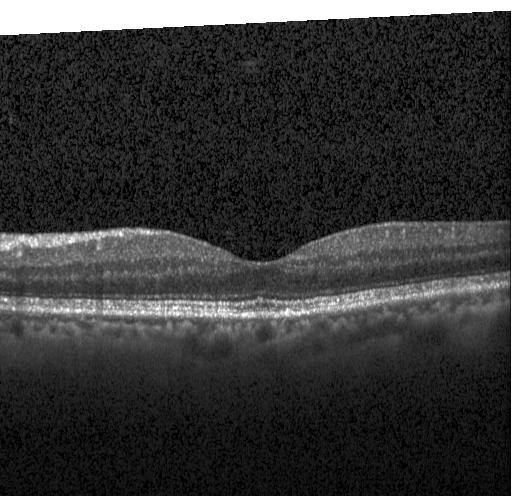
Heidelberg Spectralis · horizontal scan through the fovea · retinal OCT B-scan.
Finding: no evidence of choroidal neovascularization, diabetic macular edema, or drusen.